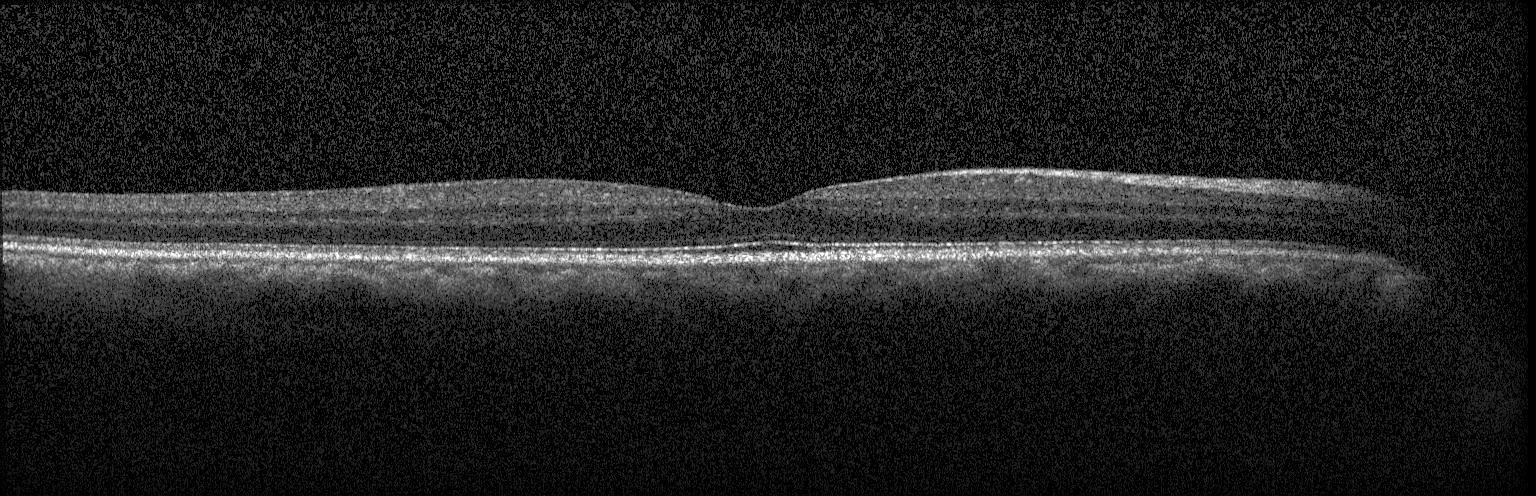 Macular OCT: no evidence of choroidal neovascularization, diabetic macular edema, or drusen.